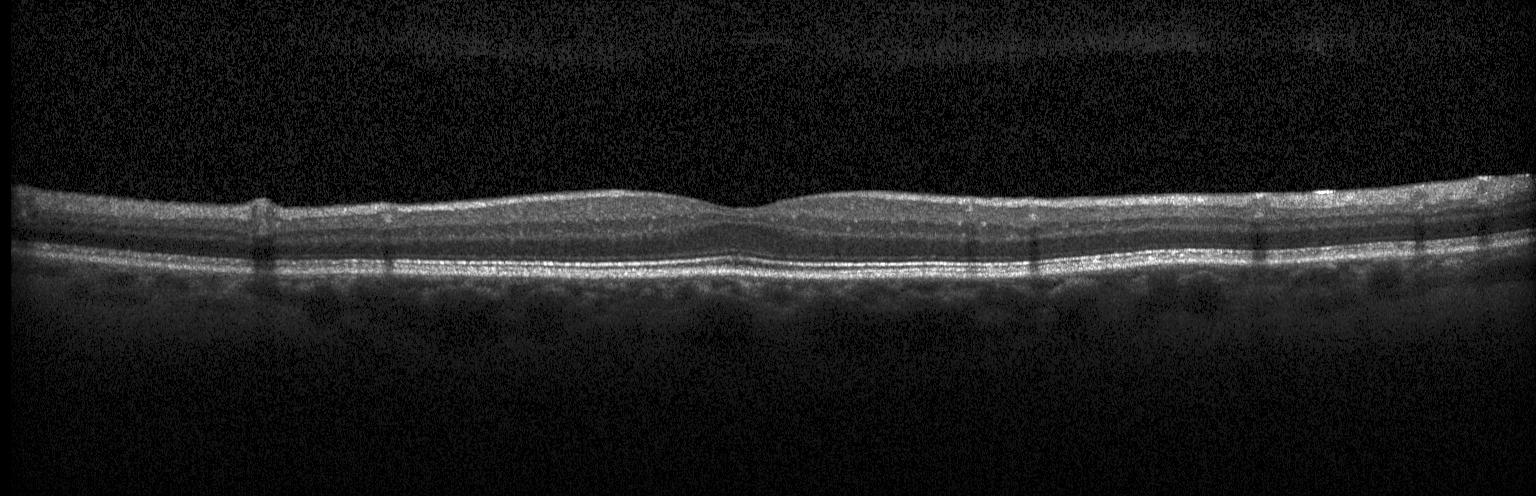

Diagnosis: neither choroidal neovascularization, diabetic macular edema, nor drusen.